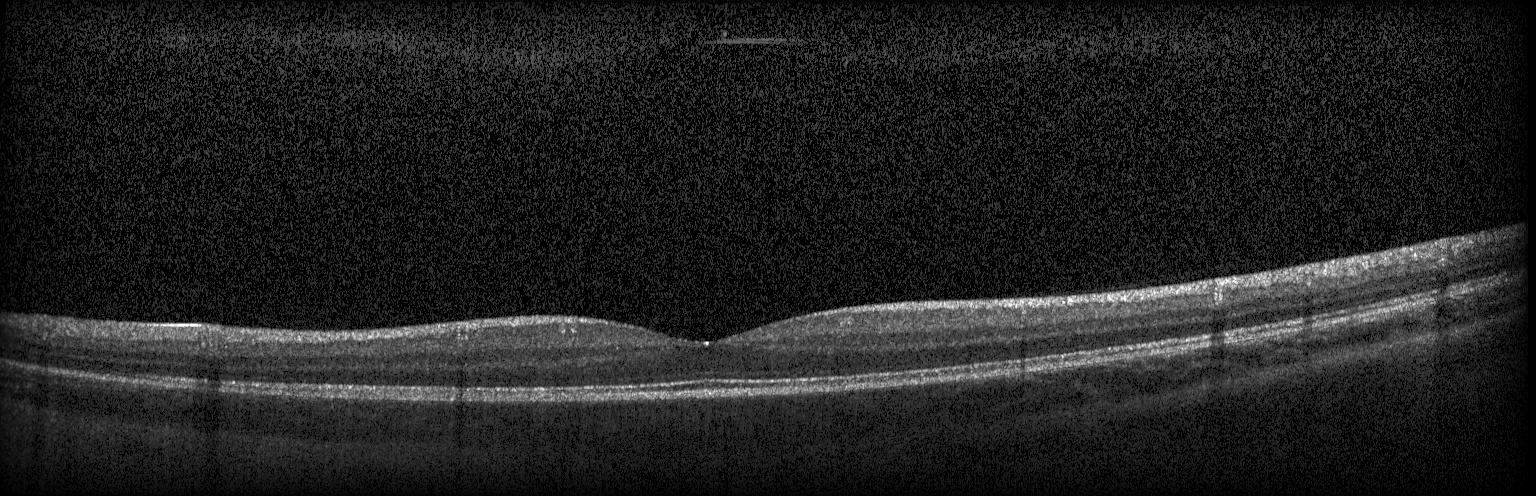
Impression: neither CNV, DME, nor drusen.